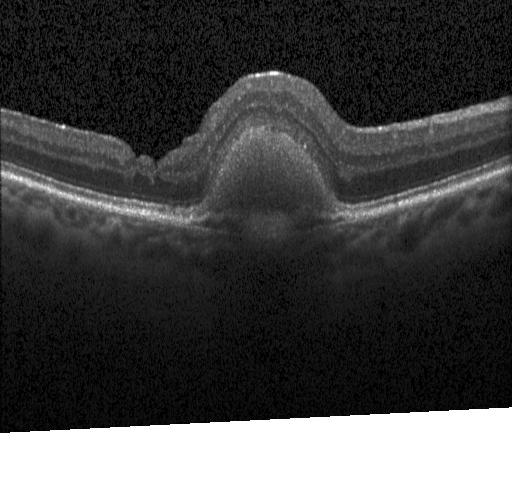

OCT scan showing choroidal neovascularization.